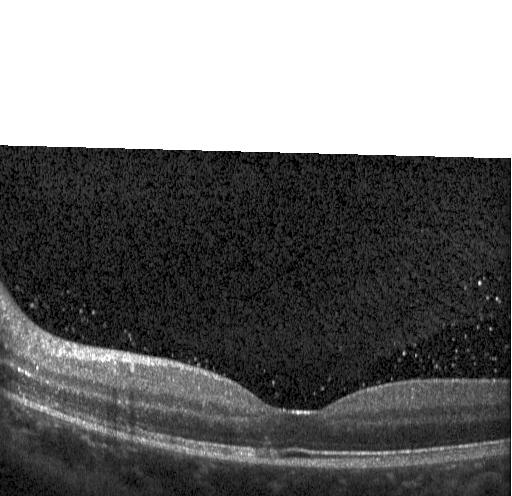 Spectral-domain optical coherence tomography; retinal OCT B-scan; Heidelberg Spectralis; through the macula.
Impression: no evidence of choroidal neovascularization, diabetic macular edema, or drusen.